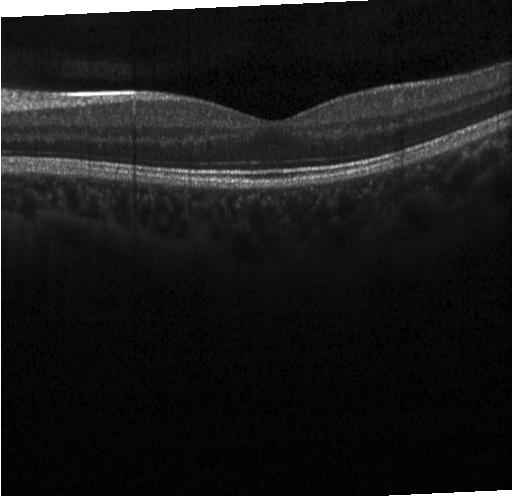

No evidence of choroidal neovascularization, diabetic macular edema, or drusen.